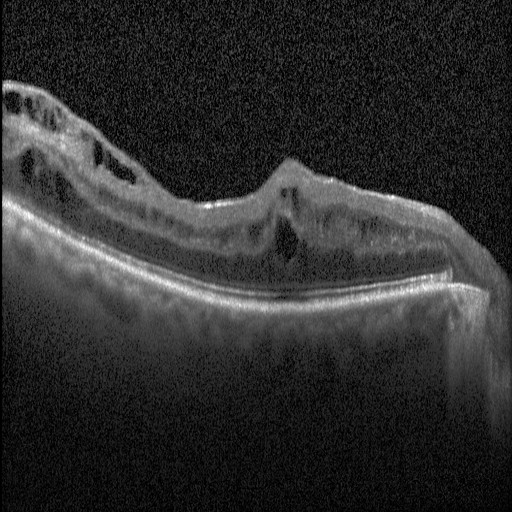

SD-OCT, acquired on a Heidelberg Spectralis, OCT line scan.
This B-scan demonstrates diabetic macular edema (DME).